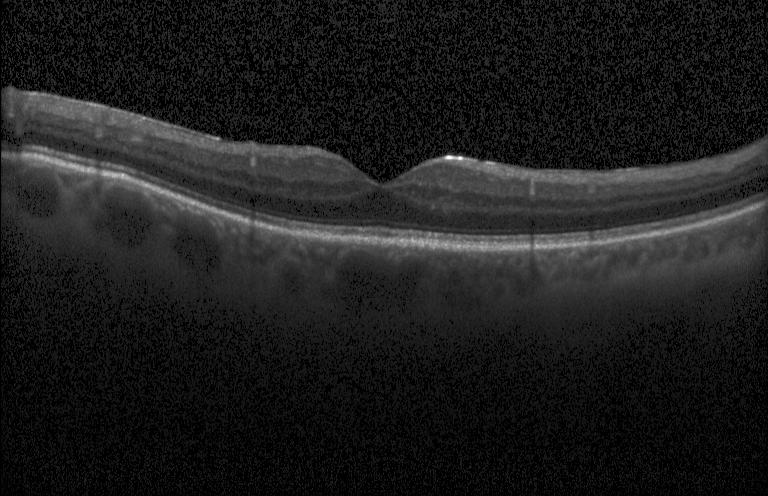 Centered on the fovea; Heidelberg Spectralis OCT system; OCT line scan.
Dx: neither choroidal neovascularization, diabetic macular edema, nor drusen.